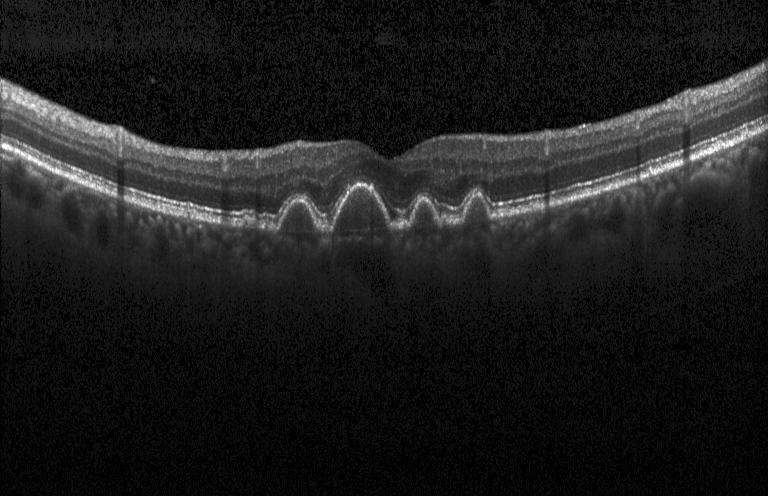
OCT B-scan. Finding: sub-RPE drusenoid deposits.